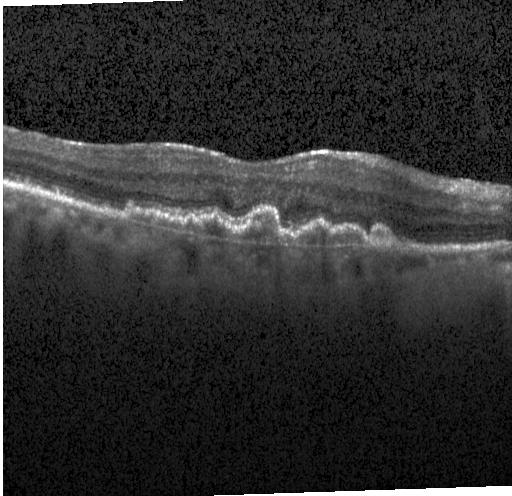

Finding: a choroidal neovascular membrane.